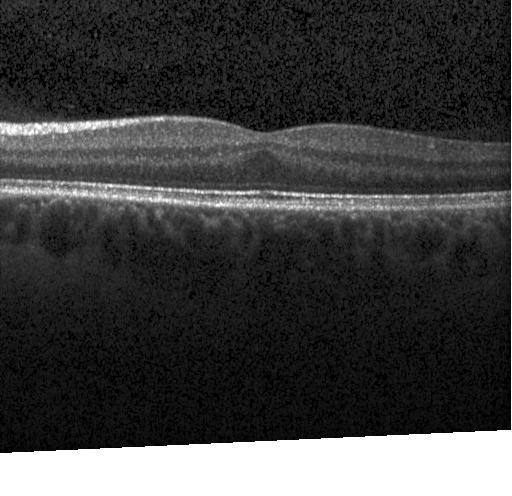 Spectral-domain OCT; fovea-centered; Heidelberg Spectralis OCT system; retinal OCT B-scan.
OCT finding: no choroidal neovascularization, no diabetic macular edema, and no drusen.